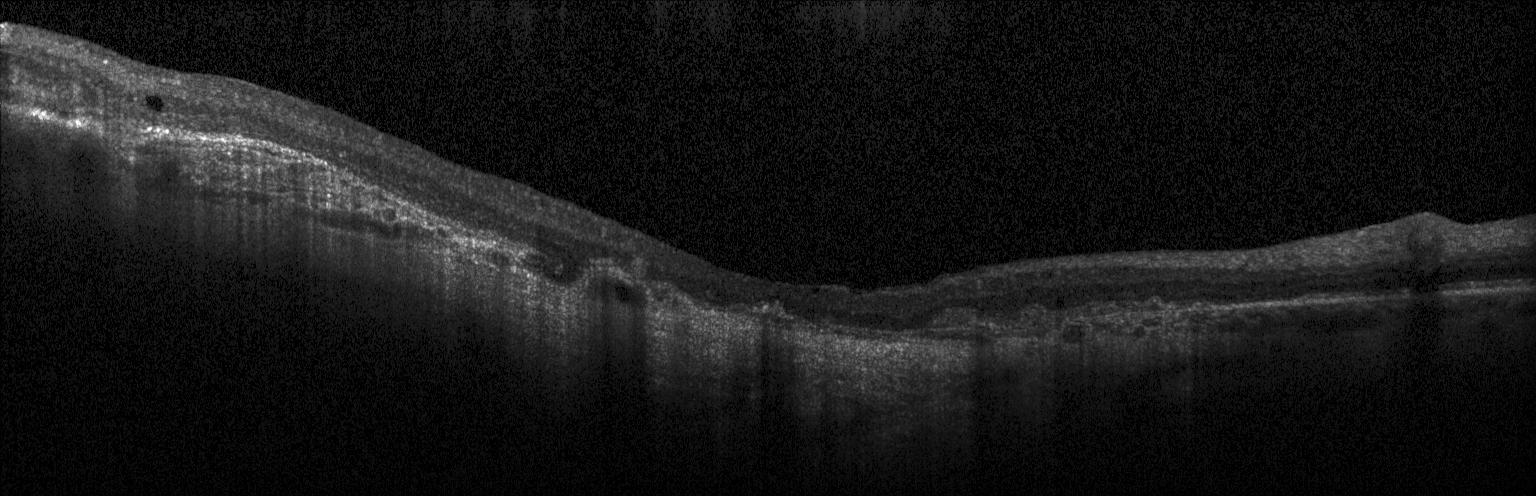

Fovea-centered; optical coherence tomography scan; SD-OCT. Finding: a choroidal neovascular membrane.